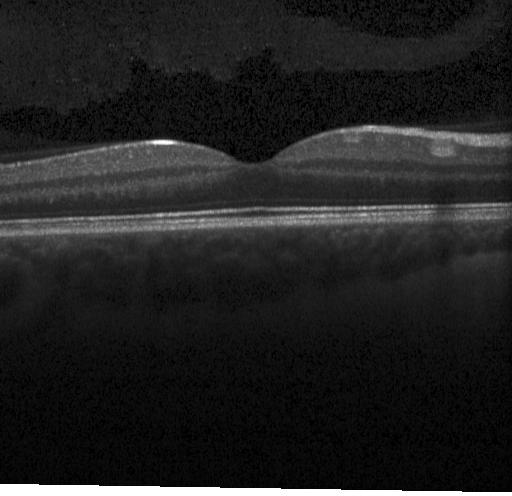 Fovea-centered, retinal OCT cross-section. Diagnosis: neither choroidal neovascularization, diabetic macular edema, nor drusen.